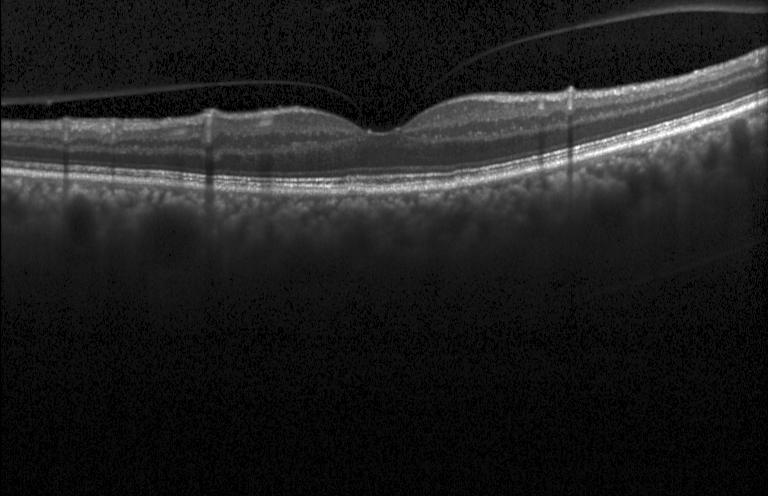
Heidelberg Spectralis OCT system; retinal OCT cross-section; centered on the fovea.
Diagnosis: neither CNV, DME, nor drusen.